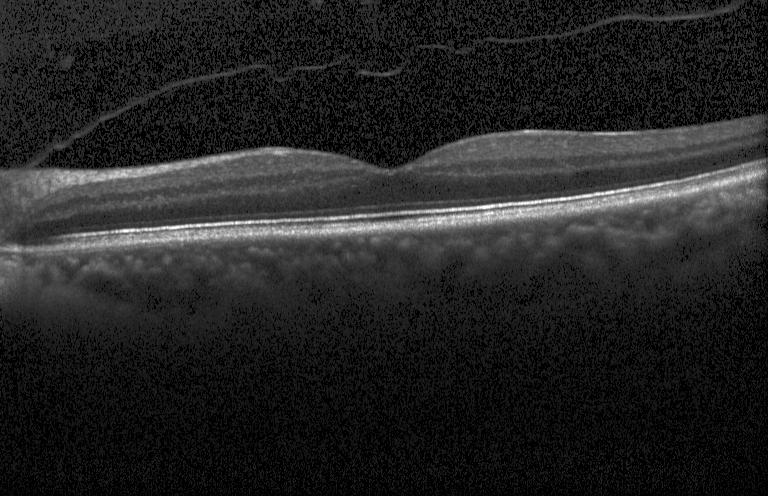 OCT B-scan, instrument: Heidelberg Spectralis, SD-OCT. Diagnosis: neither choroidal neovascularization, diabetic macular edema, nor drusen.